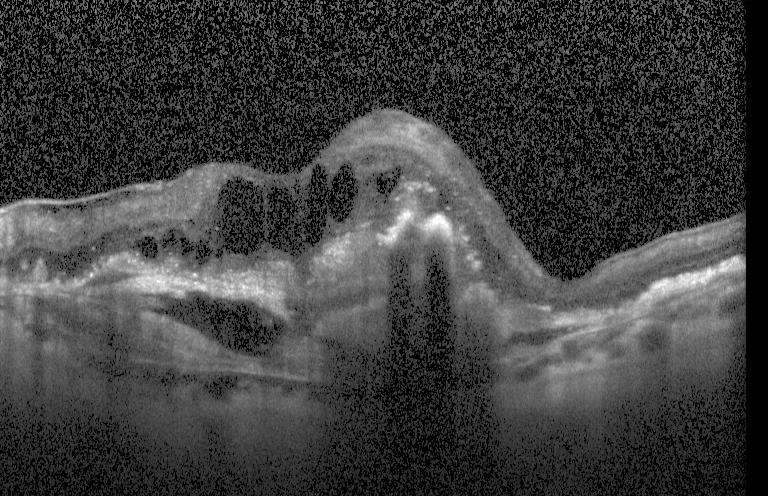 Spectral-domain OCT B-scan: a choroidal neovascular membrane.